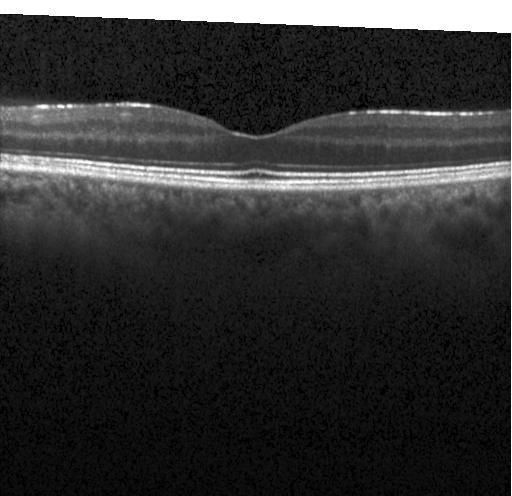 Acquired on a Heidelberg Spectralis, centered on the fovea, SD-OCT, retinal OCT B-scan. No evidence of choroidal neovascularization, diabetic macular edema, or drusen.